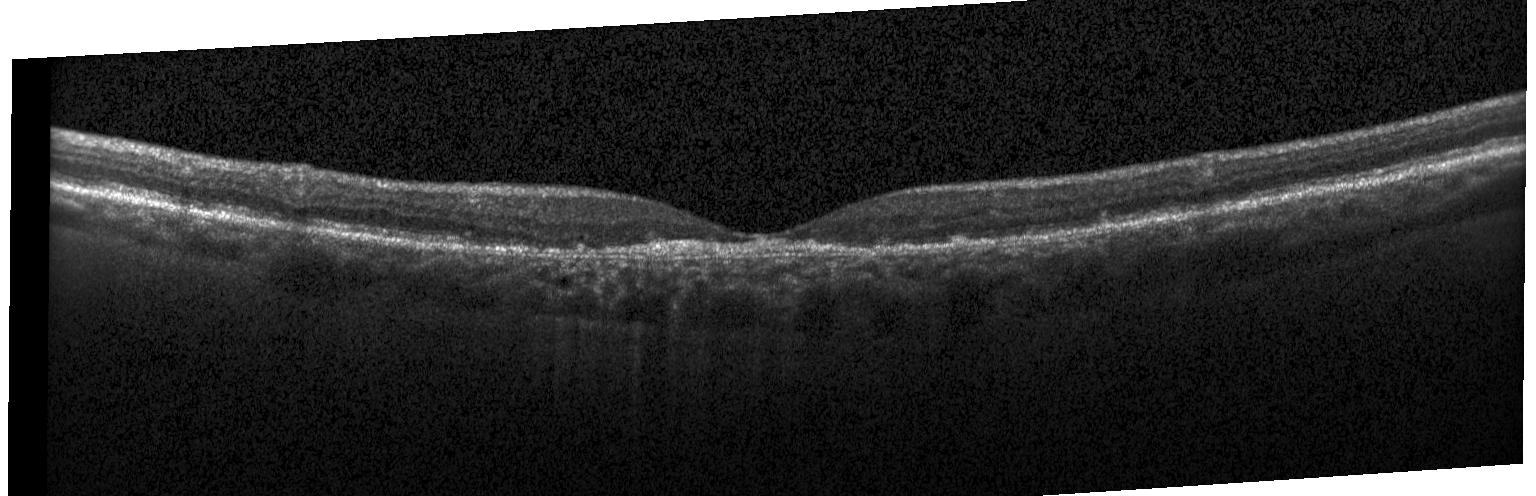

Optical coherence tomography B-scan. Heidelberg Spectralis OCT system
Finding: a choroidal neovascular membrane.